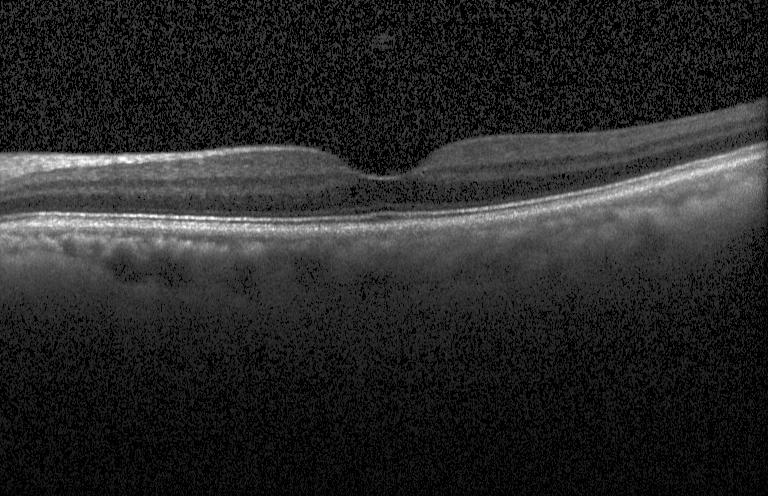
Assessment: no choroidal neovascularization, diabetic macular edema, or drusen.